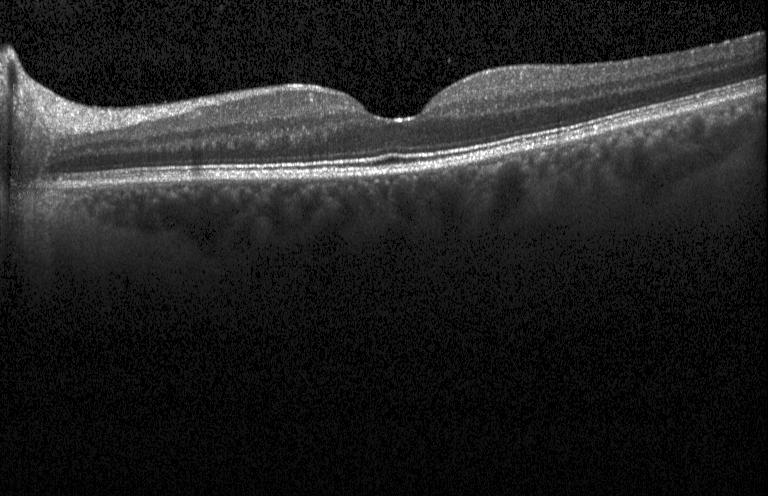
Macular scan. Optical coherence tomography scan. Heidelberg Spectralis. Spectral-domain optical coherence tomography — This B-scan demonstrates neither choroidal neovascularization, diabetic macular edema, nor drusen.